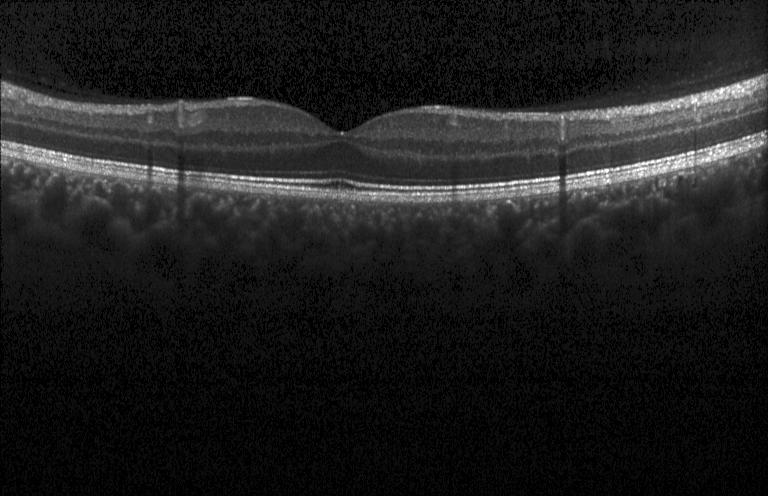

Spectral-domain optical coherence tomography · Heidelberg Spectralis · OCT B-scan · fovea-centered.
This B-scan demonstrates no choroidal neovascularization, no diabetic macular edema, and no drusen.